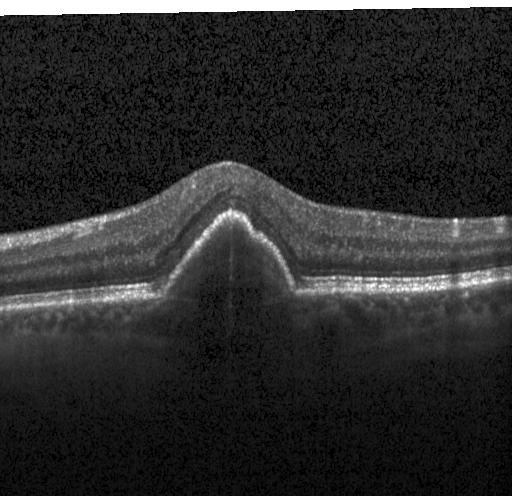

Impression: a choroidal neovascular membrane.